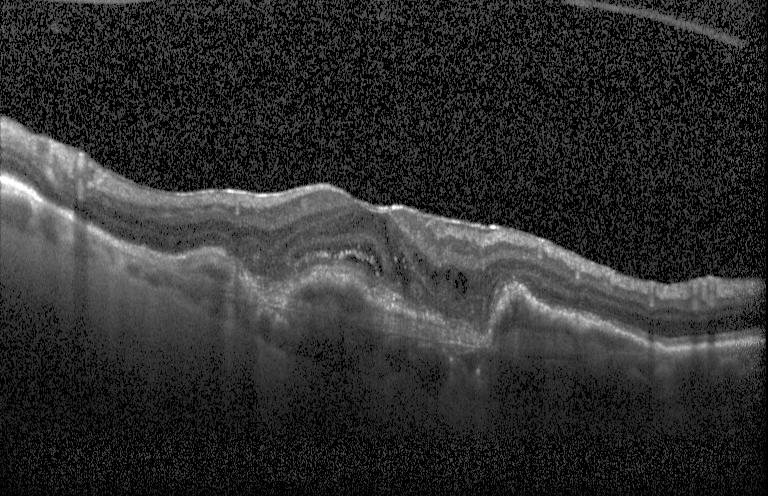
This B-scan demonstrates a choroidal neovascular membrane.